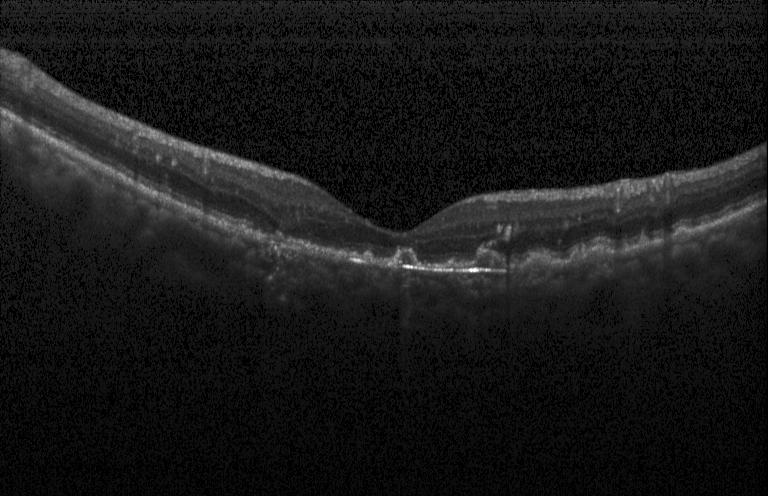
Macular scan, retinal OCT cross-section
The scan shows choroidal neovascularization.